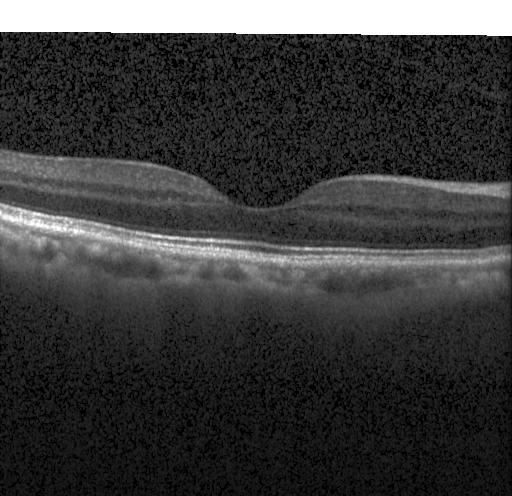

Neither CNV, DME, nor drusen.